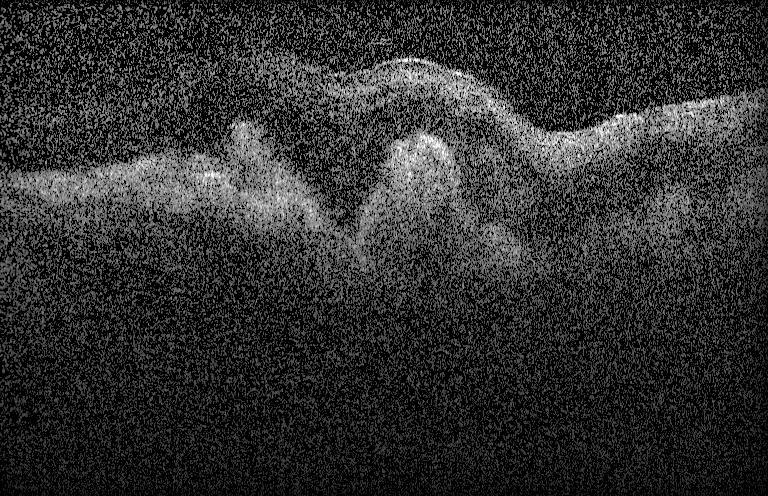
Through the macula. Heidelberg Spectralis OCT system. SD-OCT. Optical coherence tomography B-scan
Impression: choroidal neovascularization (CNV).